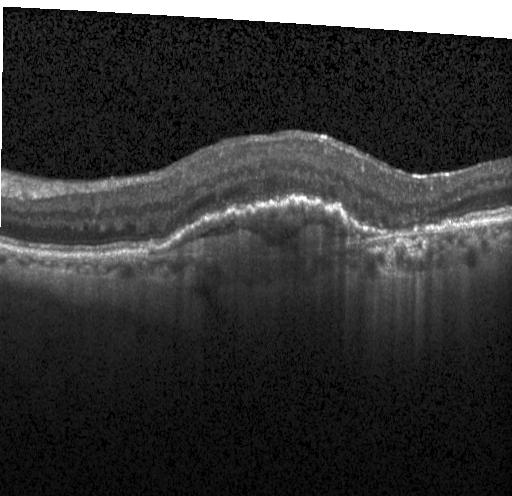 Optical coherence tomography scan
The scan shows a choroidal neovascular membrane.